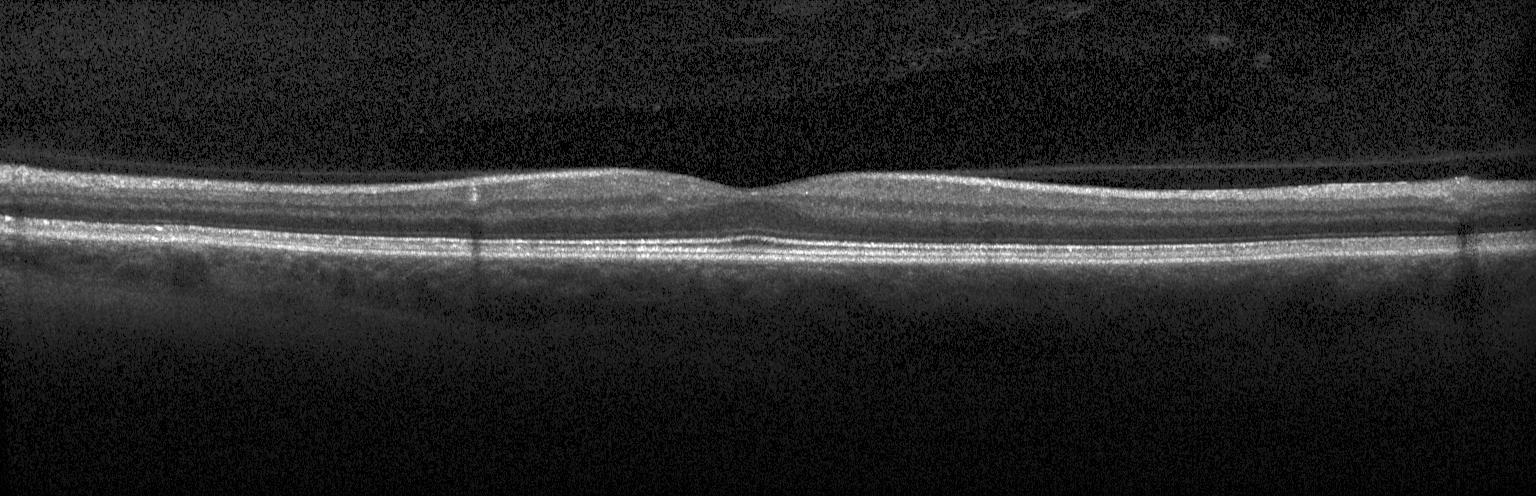
OCT finding: no choroidal neovascularization, diabetic macular edema, or drusen.